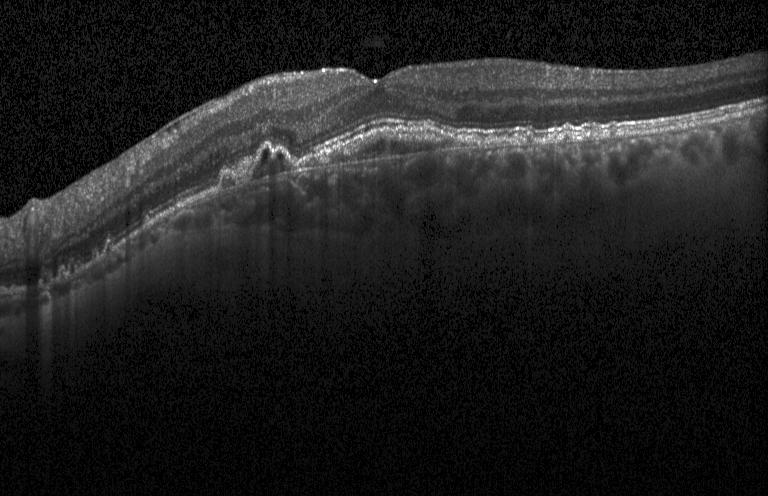 Macular scan · instrument: Heidelberg Spectralis · optical coherence tomography B-scan. Assessment: choroidal neovascularization (CNV).